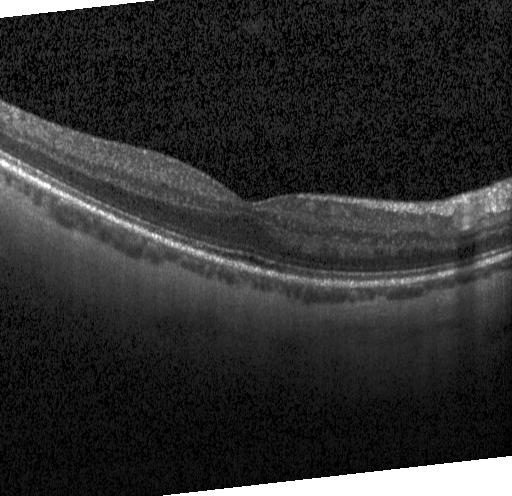
Retinal OCT B-scan. Heidelberg Spectralis. Macular scan.
Finding: no CNV, DME, or drusen.